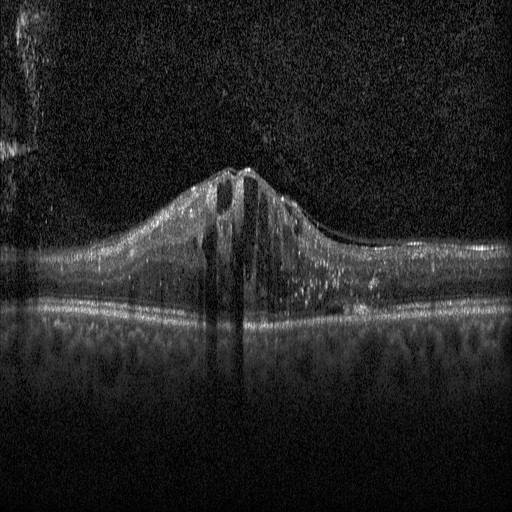 Instrument: Heidelberg Spectralis · OCT B-scan · centered on the fovea. Finding: diabetic macular edema (DME).